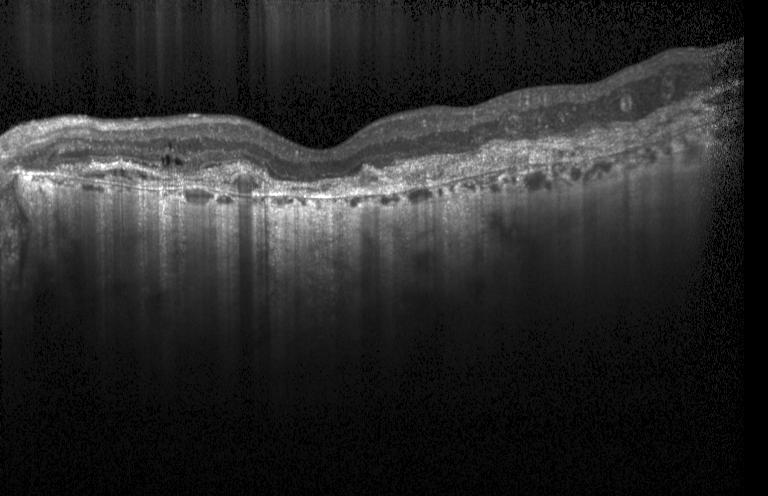 Retinal OCT B-scan. Spectral-domain optical coherence tomography. Heidelberg Spectralis OCT system
Dx: CNV.